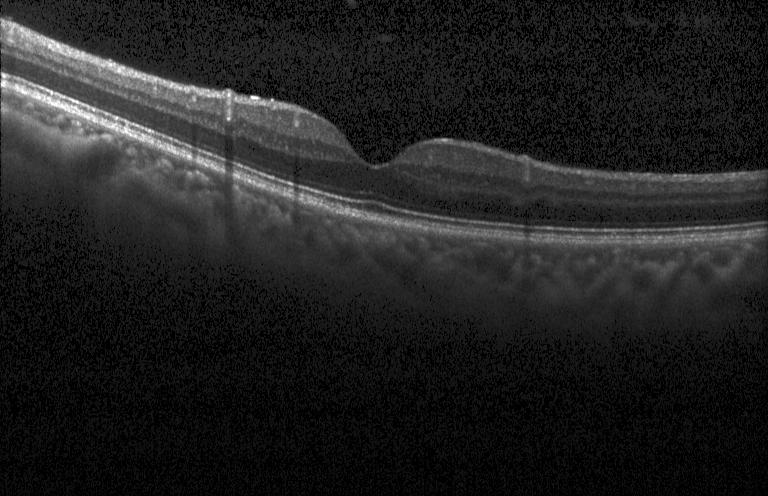
OCT B-scan showing no evidence of CNV, DME, or drusen.